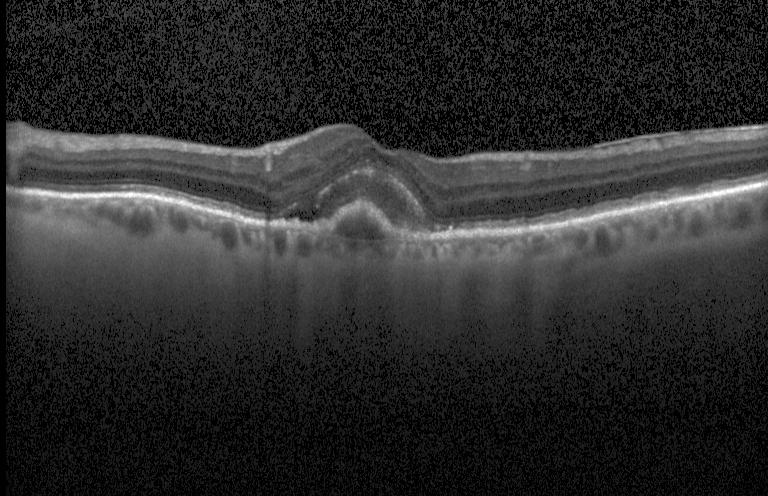
Retinal OCT cross-section — Finding: choroidal neovascularization.